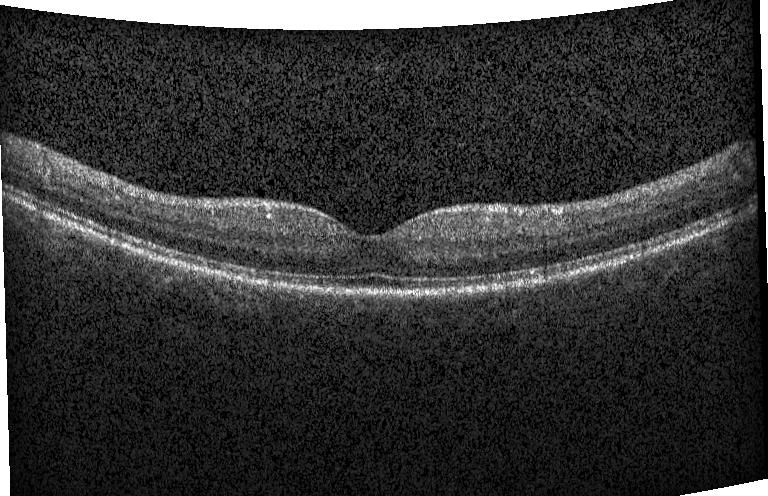

Optical coherence tomography scan
Macular OCT: no choroidal neovascularization, diabetic macular edema, or drusen.